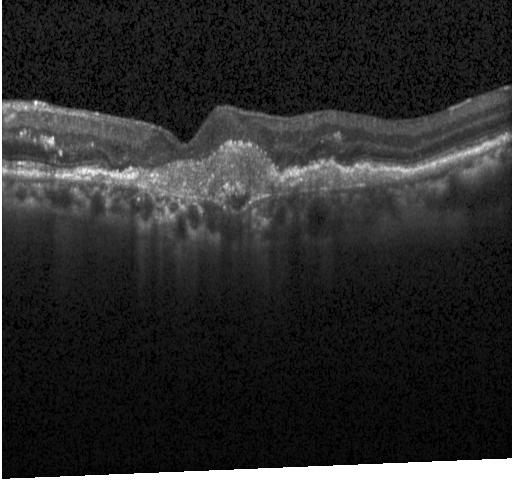 OCT B-scan showing choroidal neovascularization.